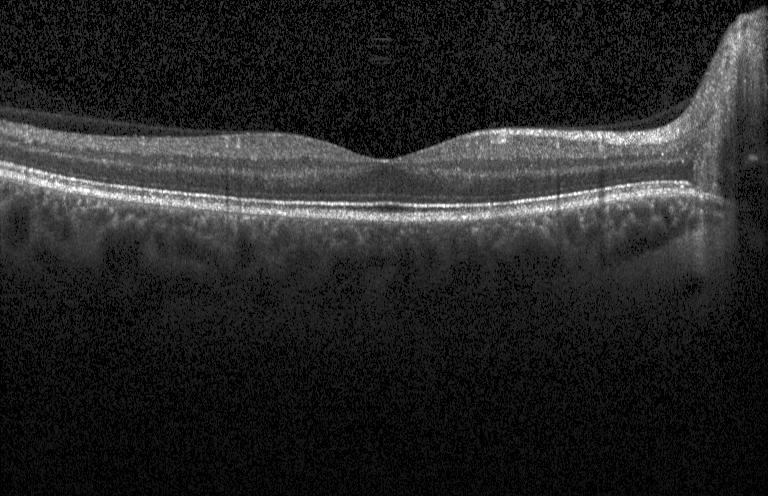
Centered on the fovea. OCT B-scan
Diagnosis: no choroidal neovascularization, no diabetic macular edema, and no drusen.